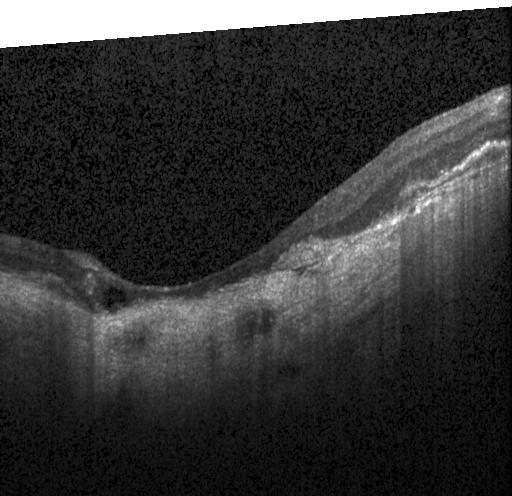
Retinal OCT cross-section — Diagnosis: choroidal neovascularization (CNV).